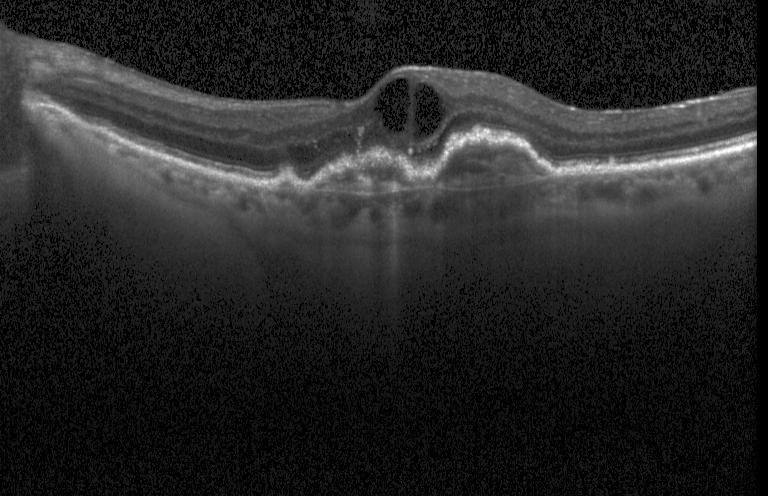 Macular scan; retinal OCT cross-section; SD-OCT — Diagnosis: a choroidal neovascular membrane.